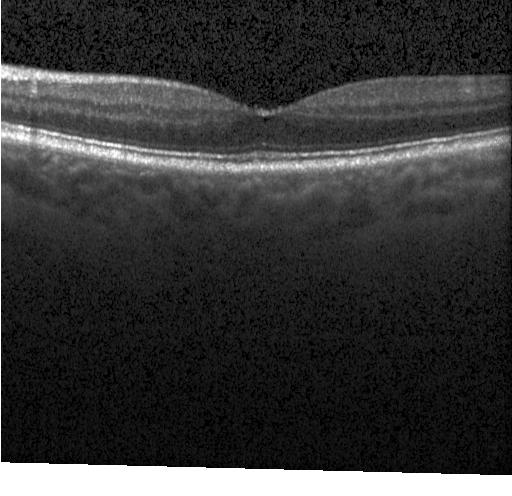

Finding: no choroidal neovascularization, no diabetic macular edema, and no drusen.